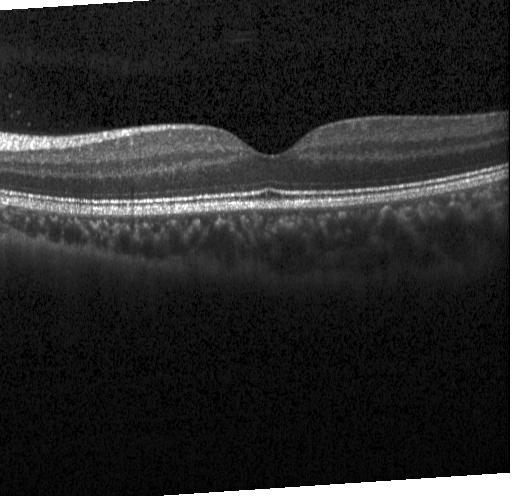

Retinal OCT cross-section.
The scan shows no evidence of CNV, DME, or drusen.